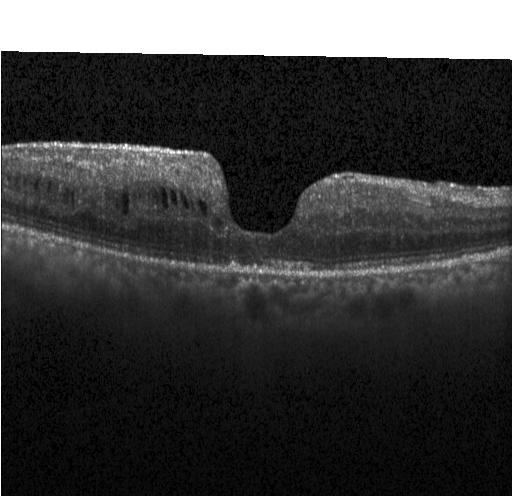 Retinal OCT B-scan.
This B-scan demonstrates diabetic macular edema.